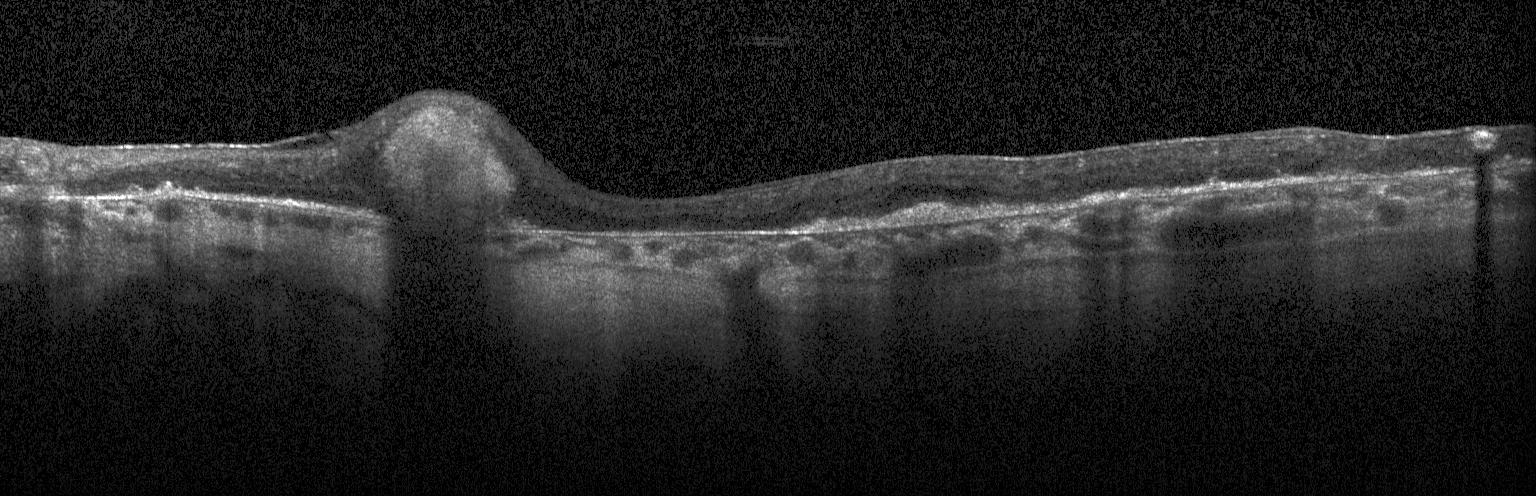 Retinal OCT B-scan; through the macula; spectral-domain OCT.
The scan shows choroidal neovascularization.